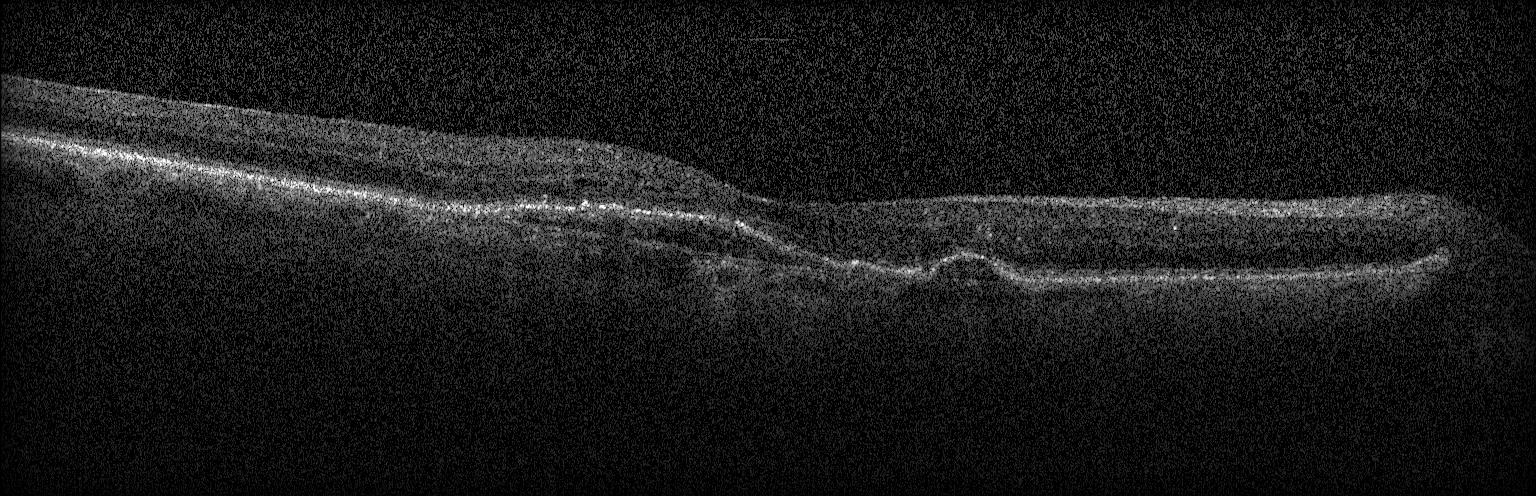

OCT line scan. Heidelberg Spectralis OCT system.
Impression: choroidal neovascularization (CNV).